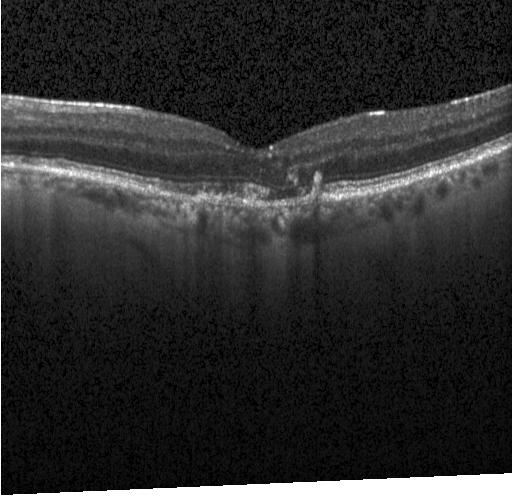

Optical coherence tomography scan. Through the macula. SD-OCT.
OCT finding: CNV.